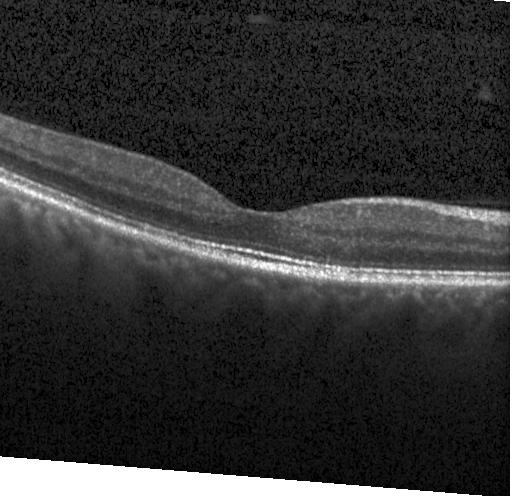

Through the macula; OCT line scan; acquired on a Heidelberg Spectralis; SD-OCT — This B-scan demonstrates neither choroidal neovascularization, diabetic macular edema, nor drusen.